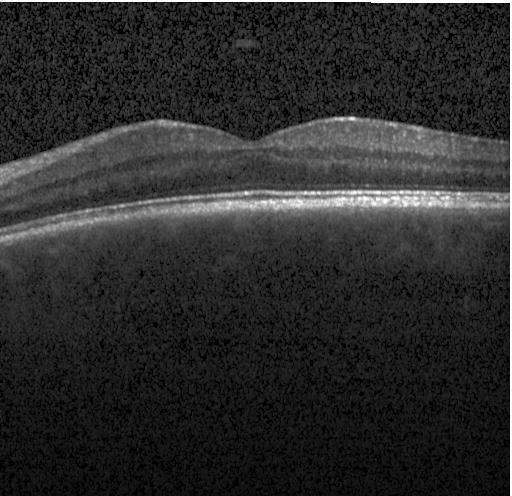

Finding: neither CNV, DME, nor drusen.